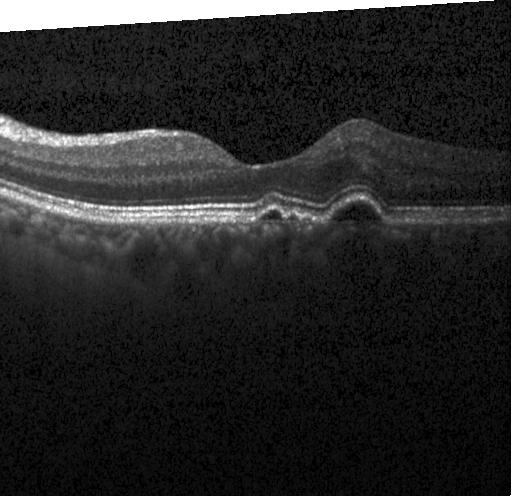

Retinal OCT cross-section · macular scan.
Diagnosis: choroidal neovascularization.